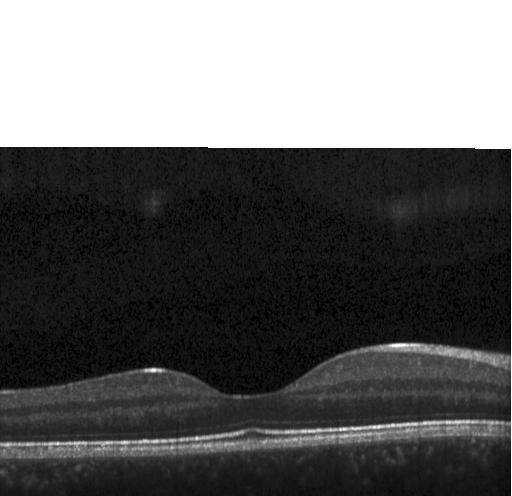
Retinal OCT B-scan.
Diagnosis: no evidence of CNV, DME, or drusen.